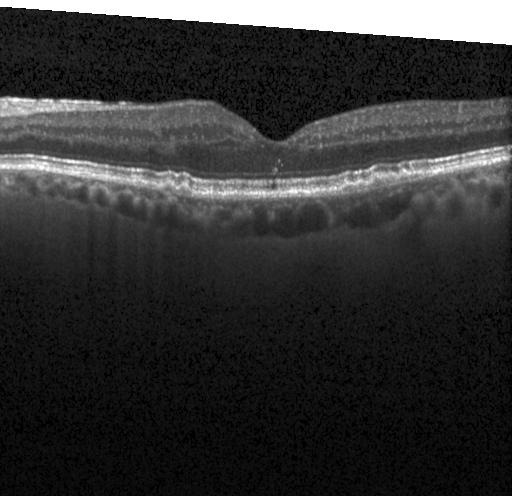 Heidelberg Spectralis OCT system · through the macula · optical coherence tomography scan · spectral-domain optical coherence tomography.
Macular OCT: drusen.